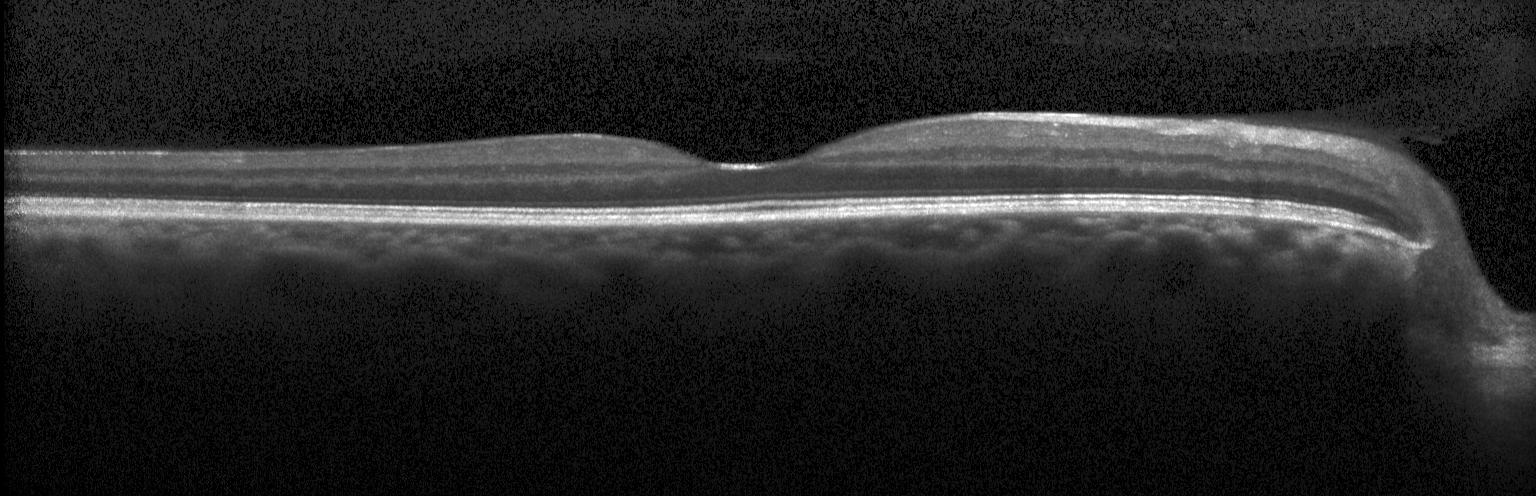
The scan shows no evidence of CNV, DME, or drusen.